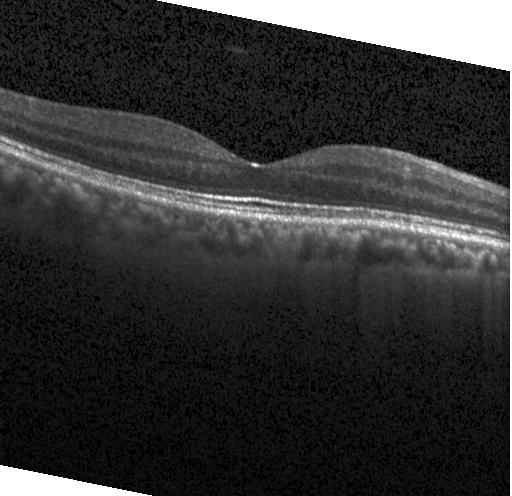 Dx: no evidence of choroidal neovascularization, diabetic macular edema, or drusen.